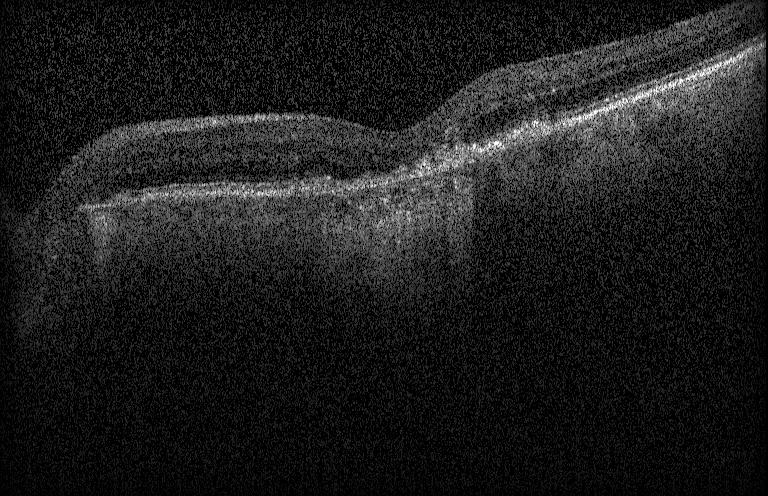

Retinal OCT B-scan · Heidelberg Spectralis · through the macula.
This B-scan demonstrates a choroidal neovascular membrane.